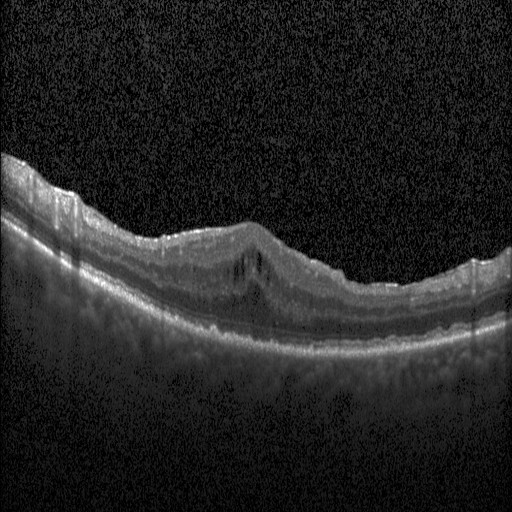 This B-scan demonstrates diabetic macular edema (DME).